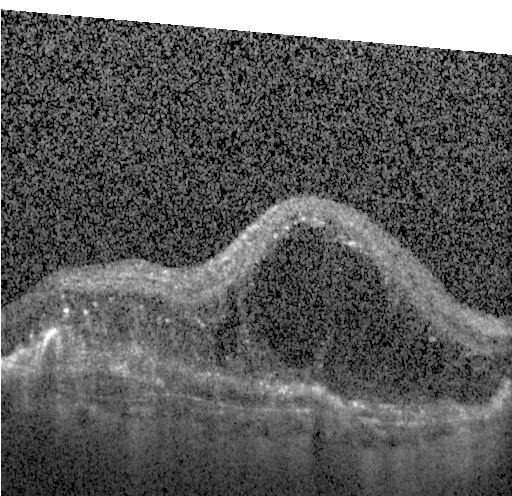

OCT B-scan. Macular OCT: a choroidal neovascular membrane.